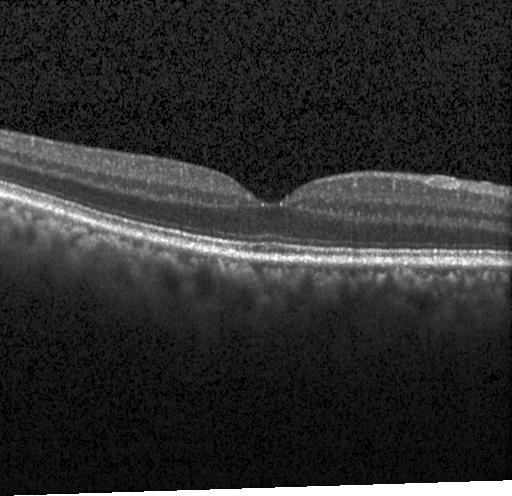
Retinal OCT B-scan
Impression: neither choroidal neovascularization, diabetic macular edema, nor drusen.